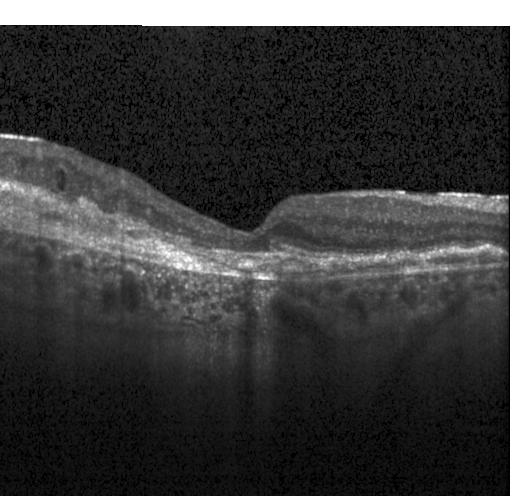

Optical coherence tomography B-scan · horizontal scan through the fovea · spectral-domain optical coherence tomography.
This B-scan demonstrates a choroidal neovascular membrane.